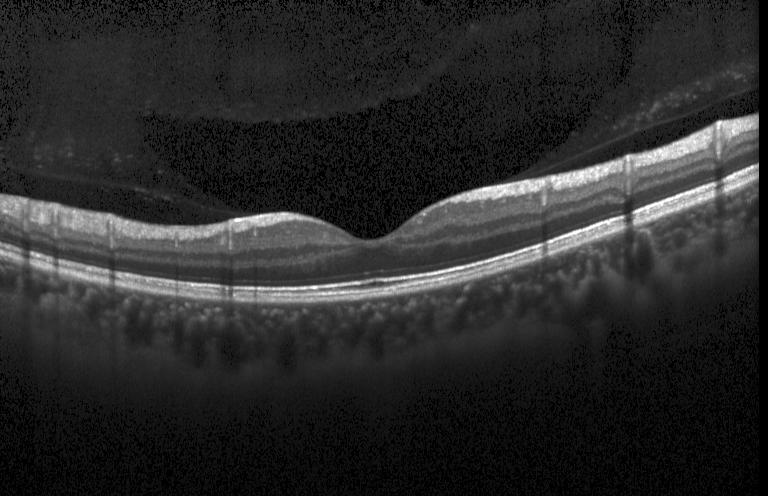
Through the macula · retinal OCT B-scan · instrument: Heidelberg Spectralis — The scan shows no evidence of choroidal neovascularization, diabetic macular edema, or drusen.